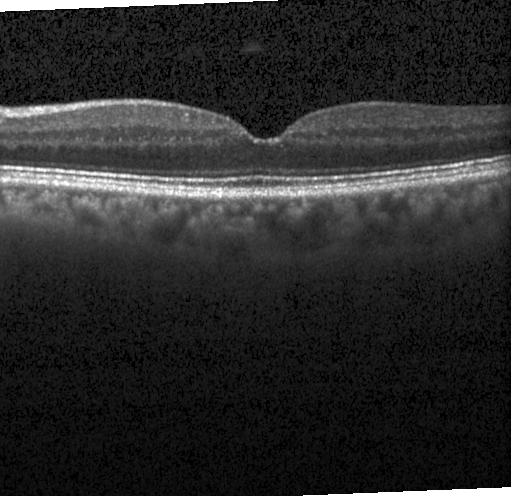

Assessment: no choroidal neovascularization, diabetic macular edema, or drusen.